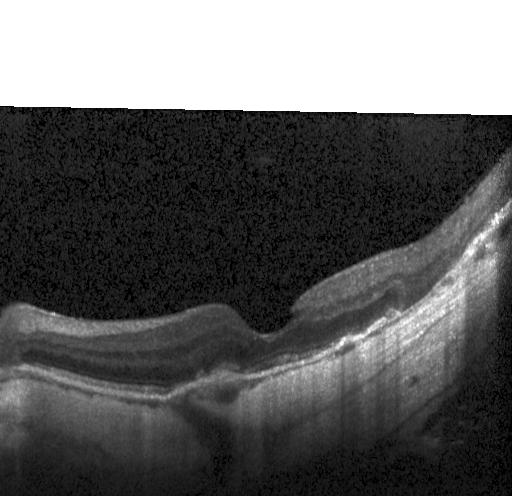 Optical coherence tomography B-scan, Heidelberg Spectralis OCT system
Finding: CNV.